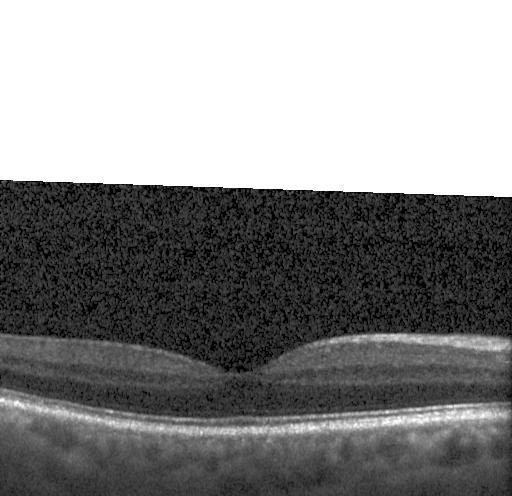
Finding: no evidence of choroidal neovascularization, diabetic macular edema, or drusen.